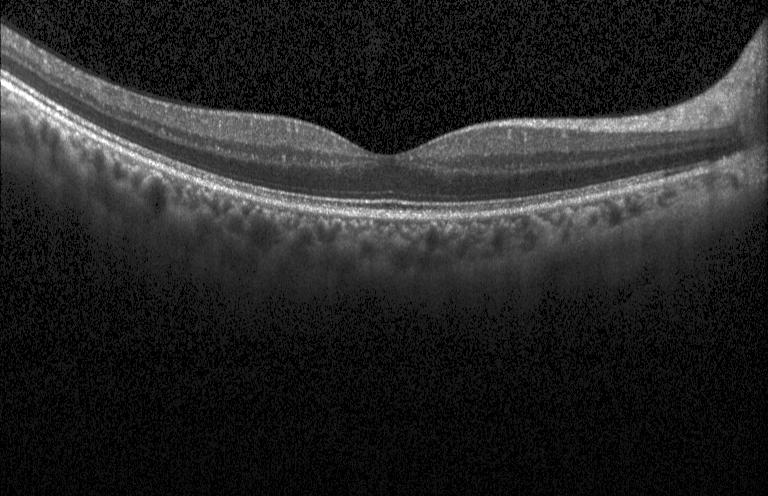

Acquired on a Heidelberg Spectralis · optical coherence tomography scan
Impression: no CNV, DME, or drusen.